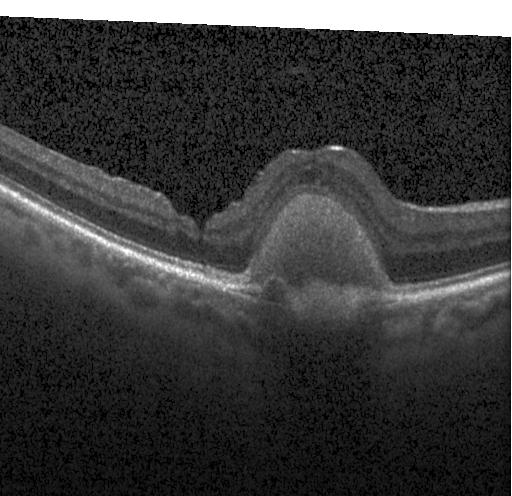 Fovea-centered · Heidelberg Spectralis · optical coherence tomography B-scan.
Diagnosis: a choroidal neovascular membrane.